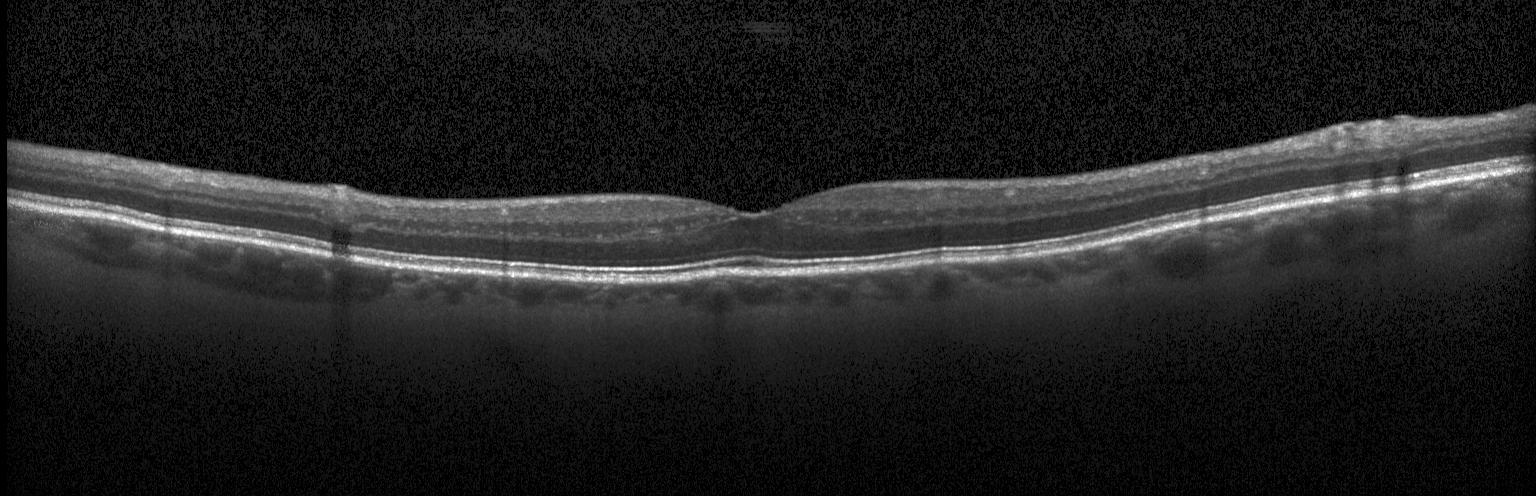
Optical coherence tomography scan · spectral-domain OCT · through the macula · Heidelberg Spectralis.
Diagnosis: neither choroidal neovascularization, diabetic macular edema, nor drusen.